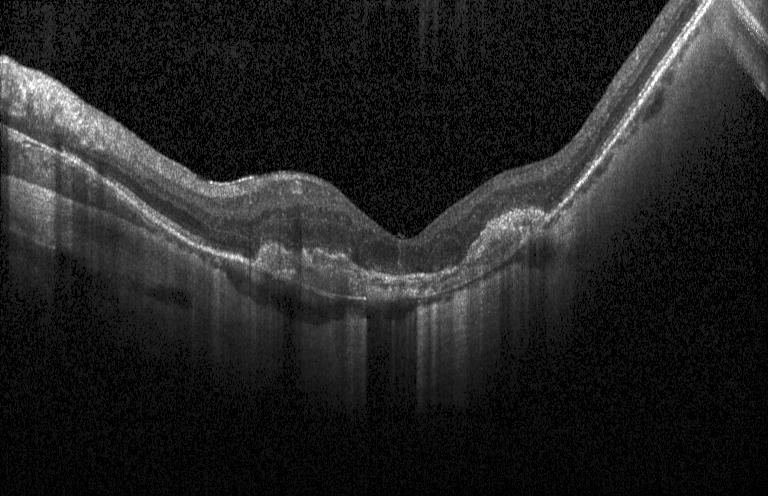

Spectral-domain OCT, instrument: Heidelberg Spectralis, macular scan, optical coherence tomography scan. Finding: a choroidal neovascular membrane.